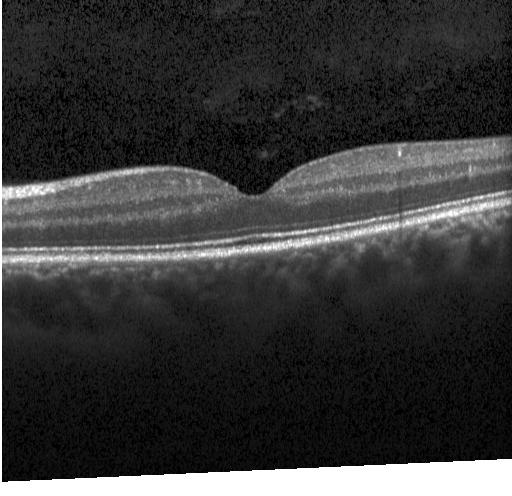 Finding: no CNV, no DME, and no drusen.